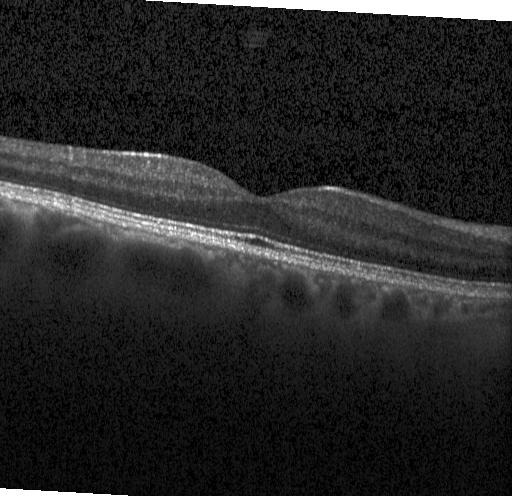
No evidence of choroidal neovascularization, diabetic macular edema, or drusen.